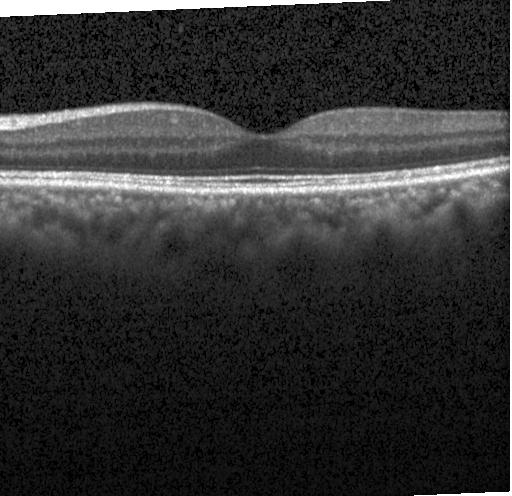
Impression: no CNV, DME, or drusen.